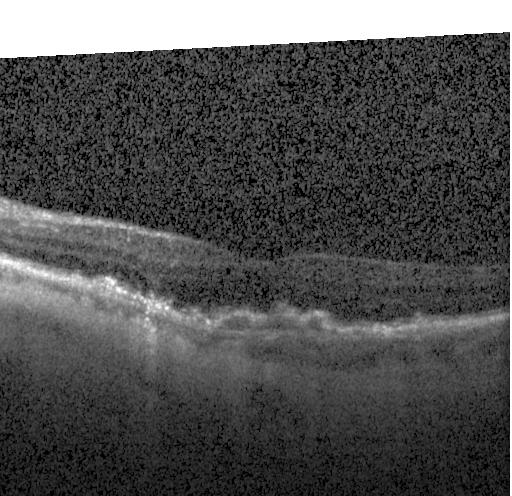

Retinal OCT cross-section
Dx: a choroidal neovascular membrane.